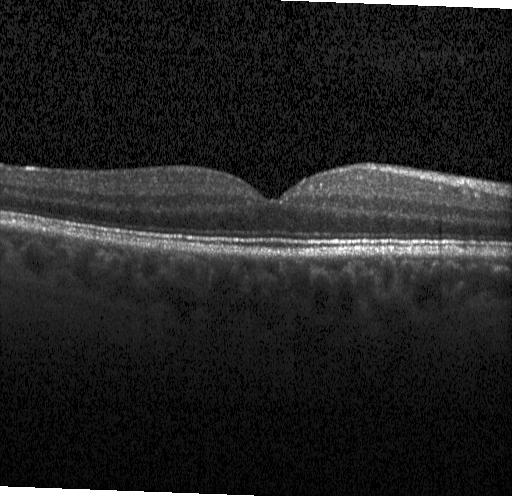 Diagnosis: no evidence of CNV, DME, or drusen.